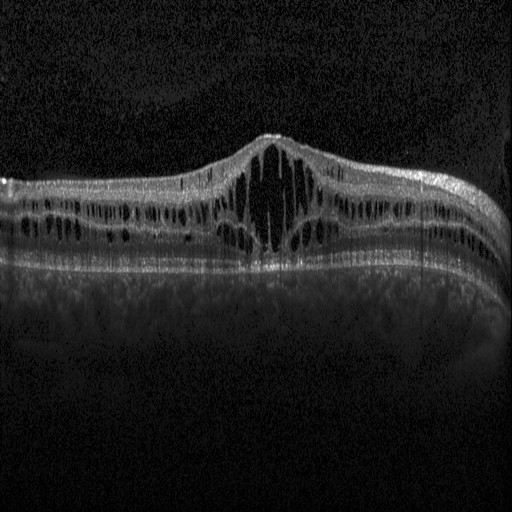
Assessment: DME.